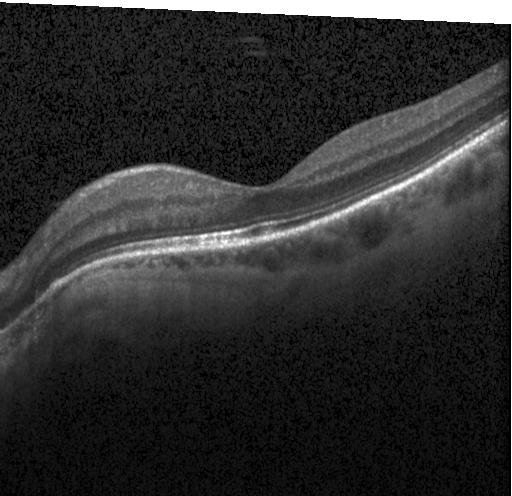 Optical coherence tomography scan, Heidelberg Spectralis OCT system.
The scan shows no choroidal neovascularization, no diabetic macular edema, and no drusen.